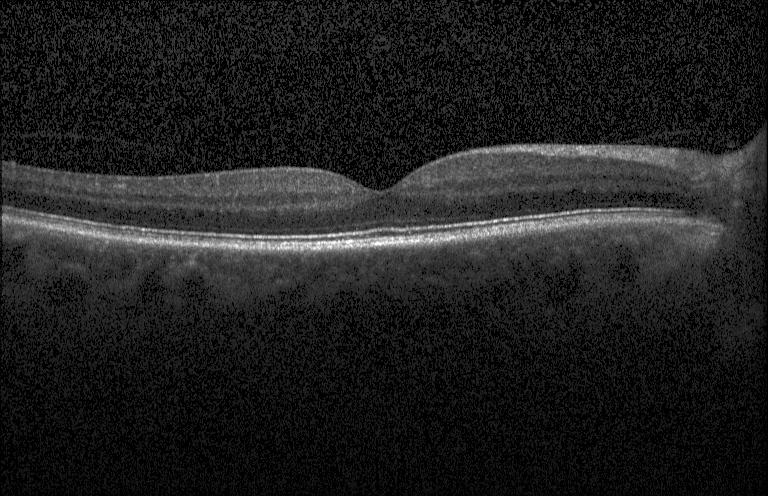 Diagnosis: no evidence of choroidal neovascularization, diabetic macular edema, or drusen.